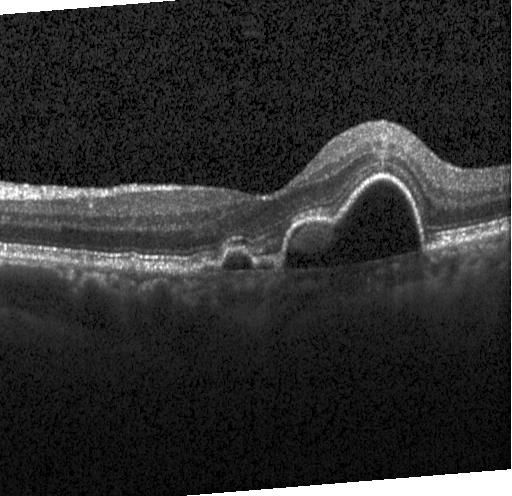 Assessment: CNV.